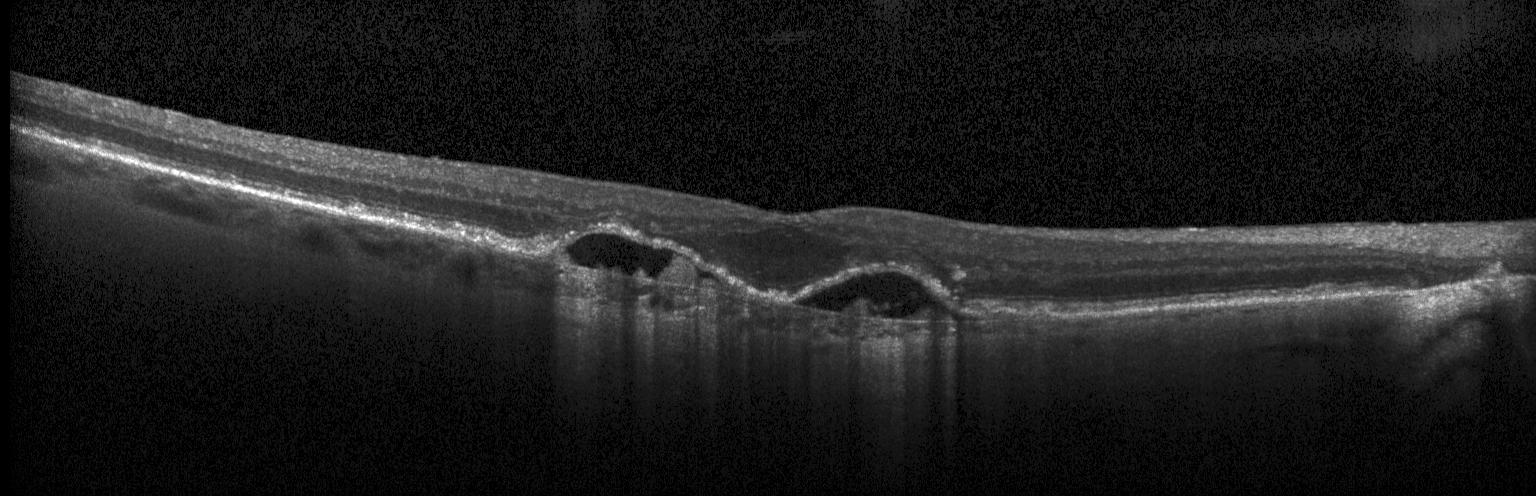
Optical coherence tomography B-scan. Instrument: Heidelberg Spectralis. Spectral-domain optical coherence tomography — Finding: choroidal neovascularization (CNV).